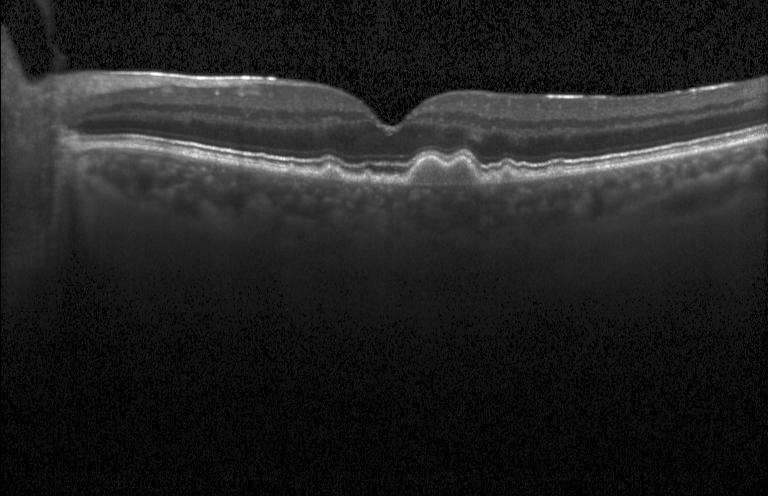
Spectral-domain OCT B-scan: drusen.